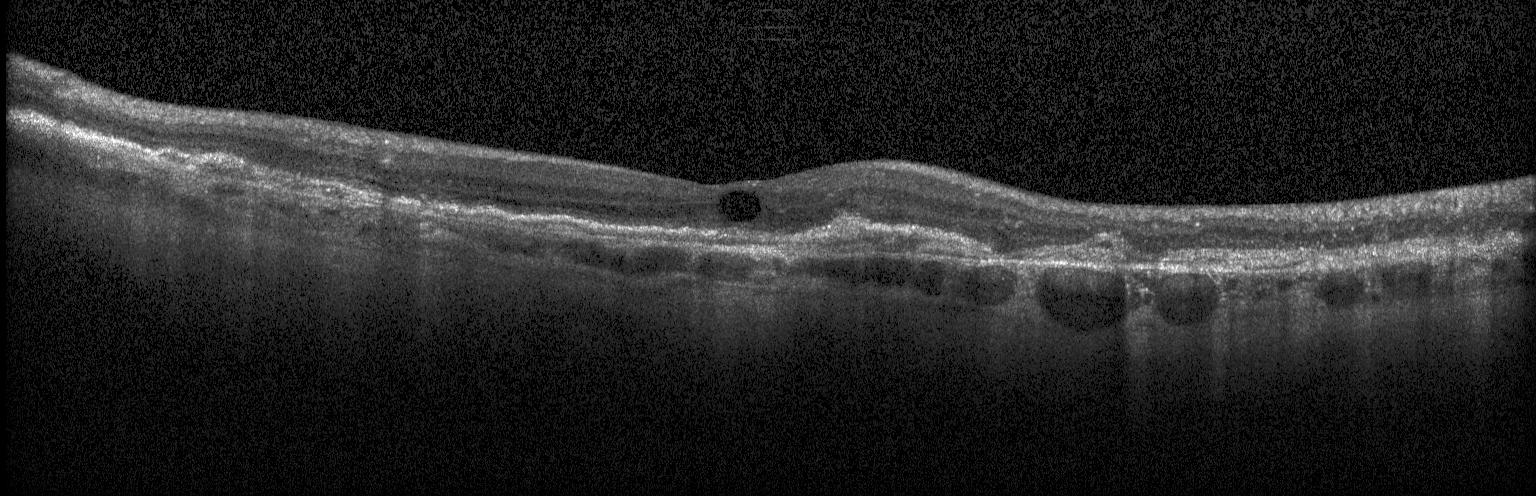 OCT B-scan. Heidelberg Spectralis OCT system
This B-scan demonstrates choroidal neovascularization.